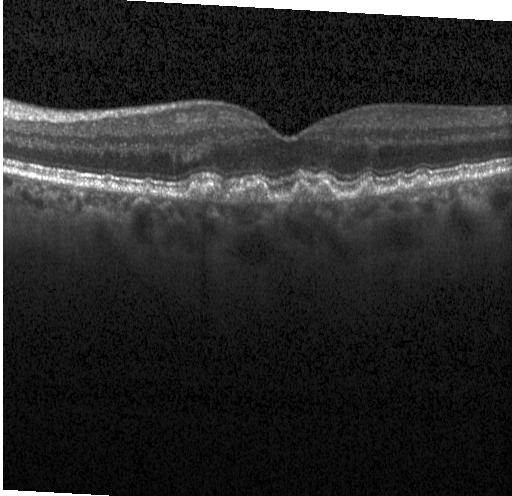 OCT line scan · through the macula
Macular OCT: multiple drusen.